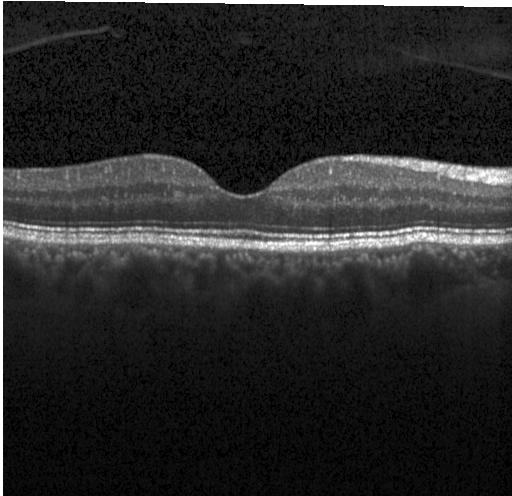 No CNV, DME, or drusen.